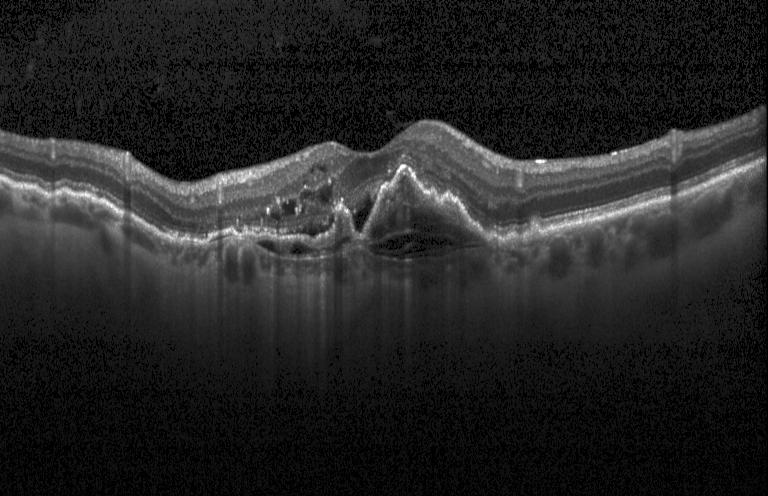

Instrument: Heidelberg Spectralis · optical coherence tomography B-scan · SD-OCT — Macular OCT: choroidal neovascularization (CNV).